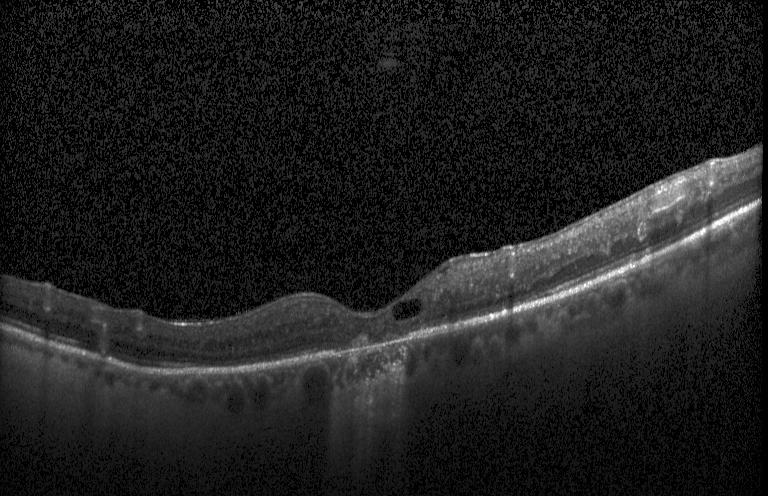

Optical coherence tomography B-scan, instrument: Heidelberg Spectralis
Dx: a choroidal neovascular membrane.